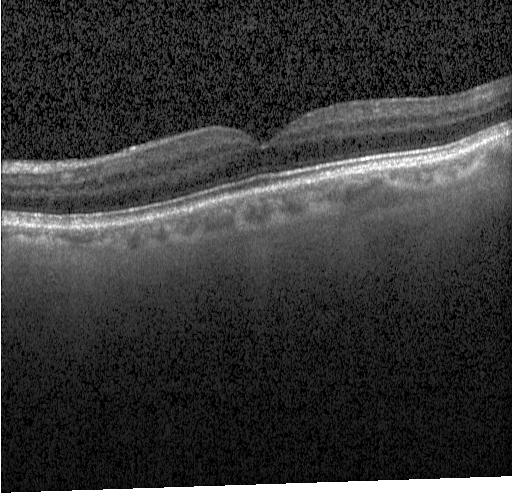

Macular OCT demonstrating neither choroidal neovascularization, diabetic macular edema, nor drusen.